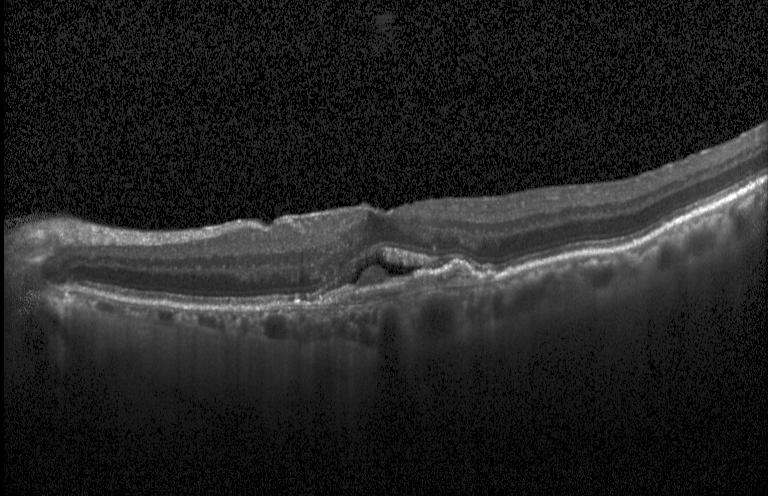

Optical coherence tomography B-scan, Heidelberg Spectralis OCT system — Impression: choroidal neovascularization.